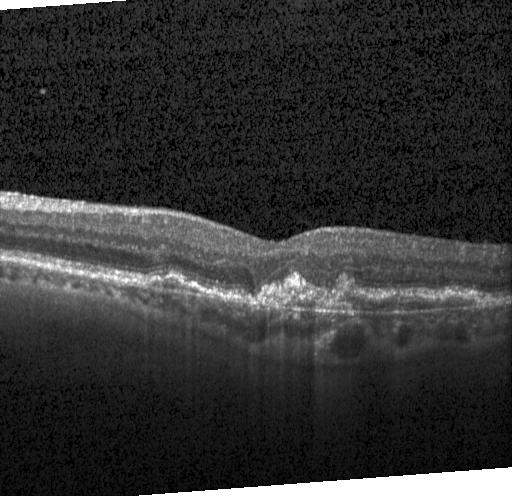
Macular OCT: a choroidal neovascular membrane.